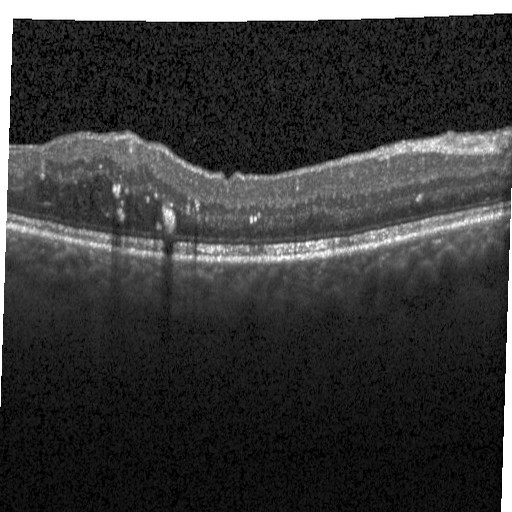
Impression: DME.